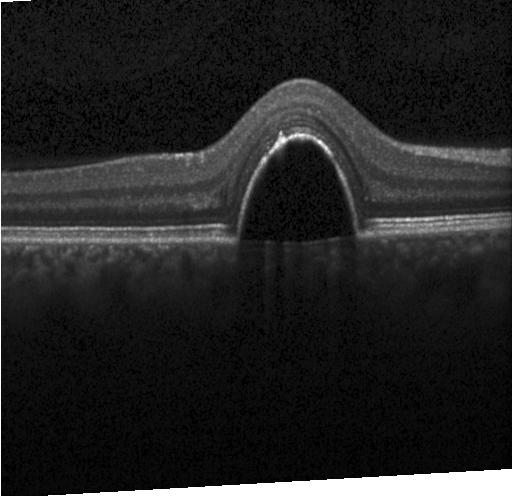

Optical coherence tomography B-scan — Choroidal neovascularization (CNV).